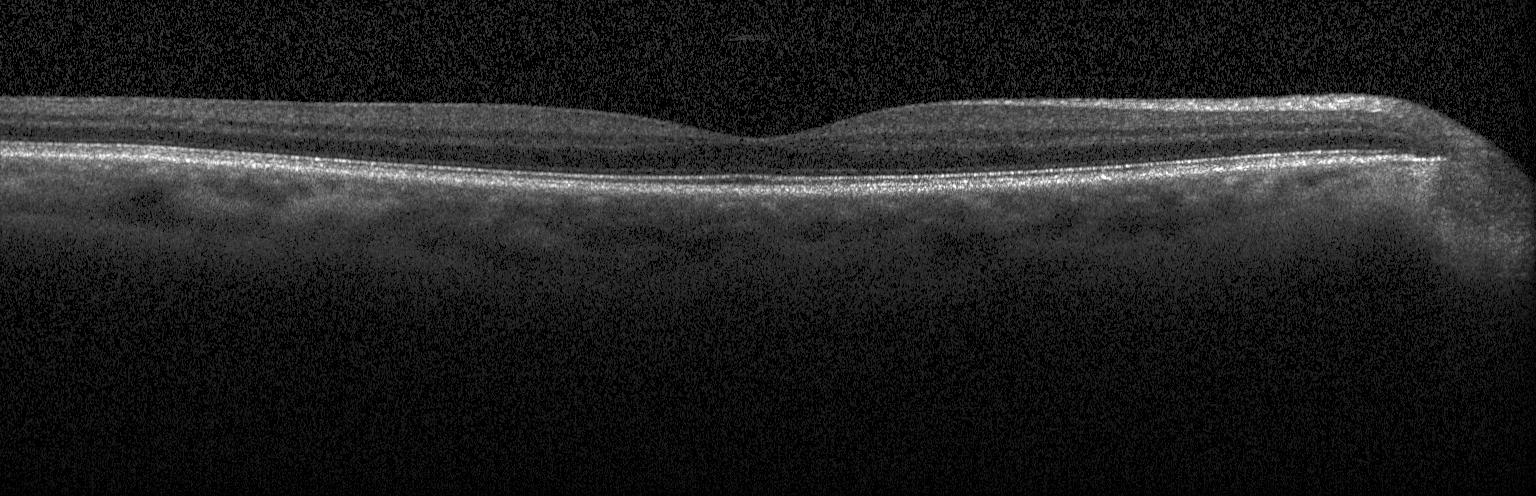 Centered on the fovea; retinal OCT B-scan; Heidelberg Spectralis.
The scan shows neither choroidal neovascularization, diabetic macular edema, nor drusen.